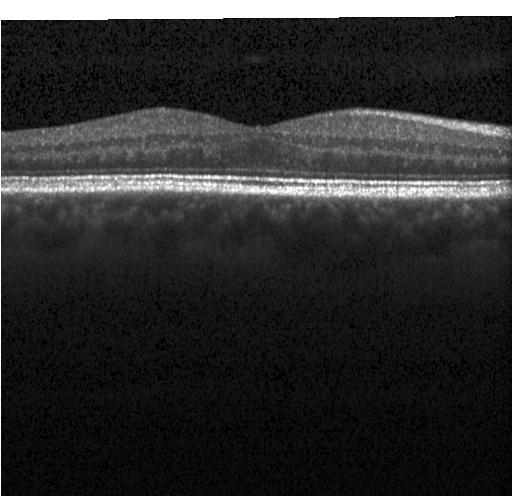
Diagnosis: no evidence of choroidal neovascularization, diabetic macular edema, or drusen.